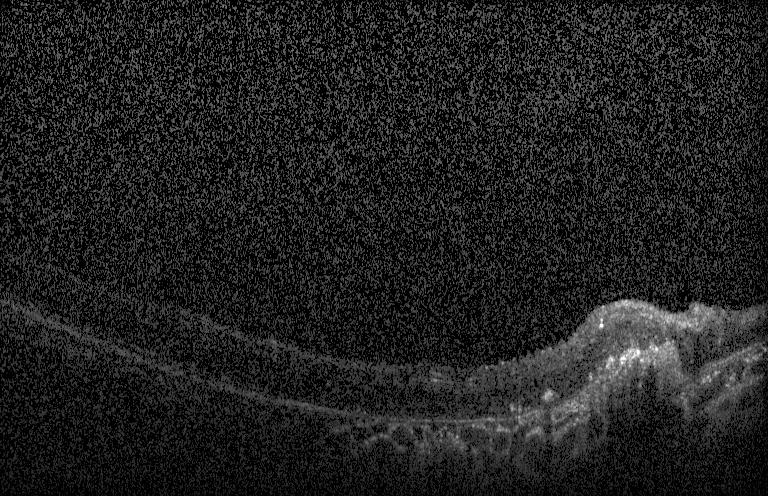 Optical coherence tomography scan; SD-OCT; instrument: Heidelberg Spectralis; horizontal scan through the fovea — This B-scan demonstrates choroidal neovascularization (CNV).